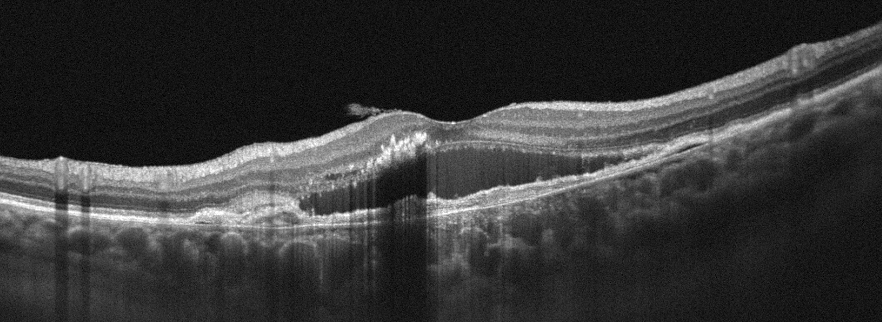 OD · OCT line scan
This B-scan demonstrates age-related macular degeneration.